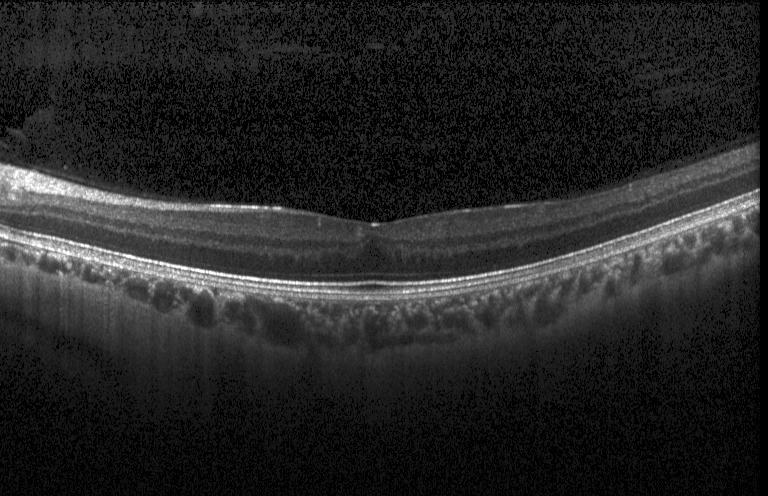

Retinal OCT B-scan, spectral-domain OCT, Heidelberg Spectralis OCT system — Finding: no evidence of choroidal neovascularization, diabetic macular edema, or drusen.